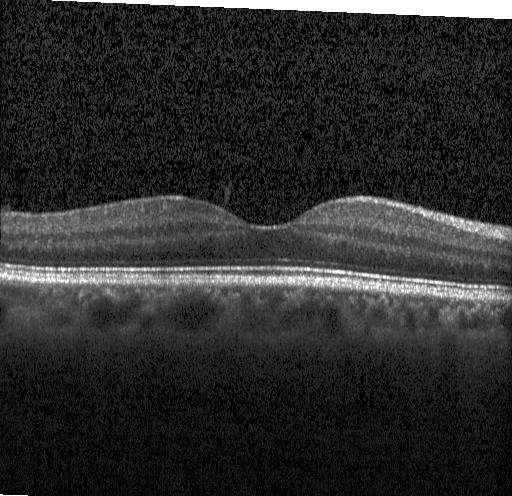

OCT B-scan · SD-OCT · acquired on a Heidelberg Spectralis.
Impression: no choroidal neovascularization, no diabetic macular edema, and no drusen.